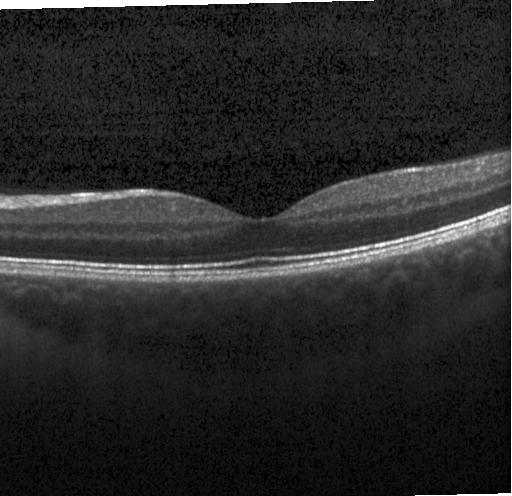 OCT B-scan, Heidelberg Spectralis OCT system
Finding: no evidence of choroidal neovascularization, diabetic macular edema, or drusen.